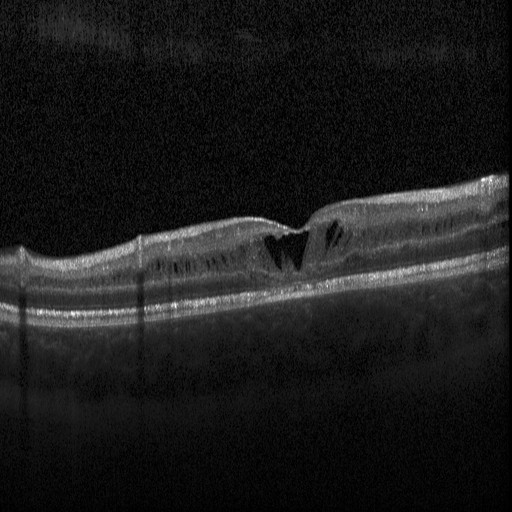 Diagnosis: diabetic macular edema (DME).